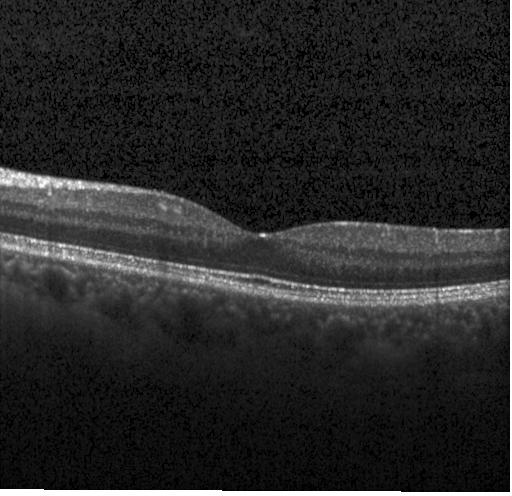
Spectral-domain OCT. Instrument: Heidelberg Spectralis. OCT line scan — Finding: neither choroidal neovascularization, diabetic macular edema, nor drusen.